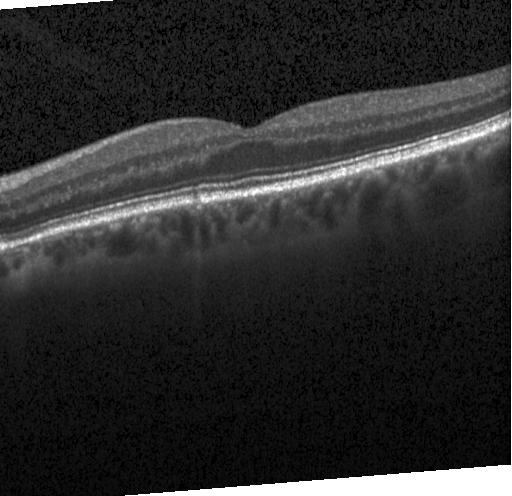 Impression: no evidence of CNV, DME, or drusen.